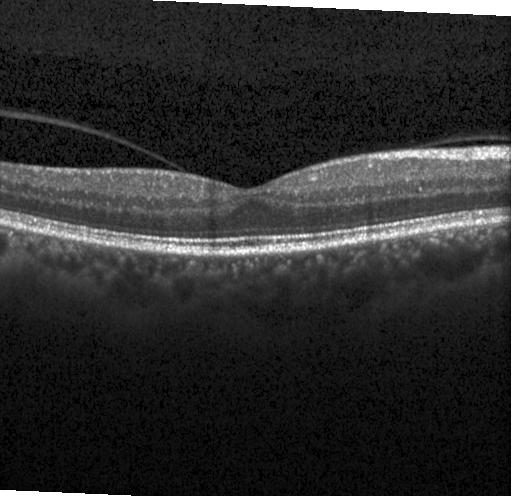

Instrument: Heidelberg Spectralis; spectral-domain optical coherence tomography; macular scan; retinal OCT B-scan
OCT finding: no choroidal neovascularization, no diabetic macular edema, and no drusen.